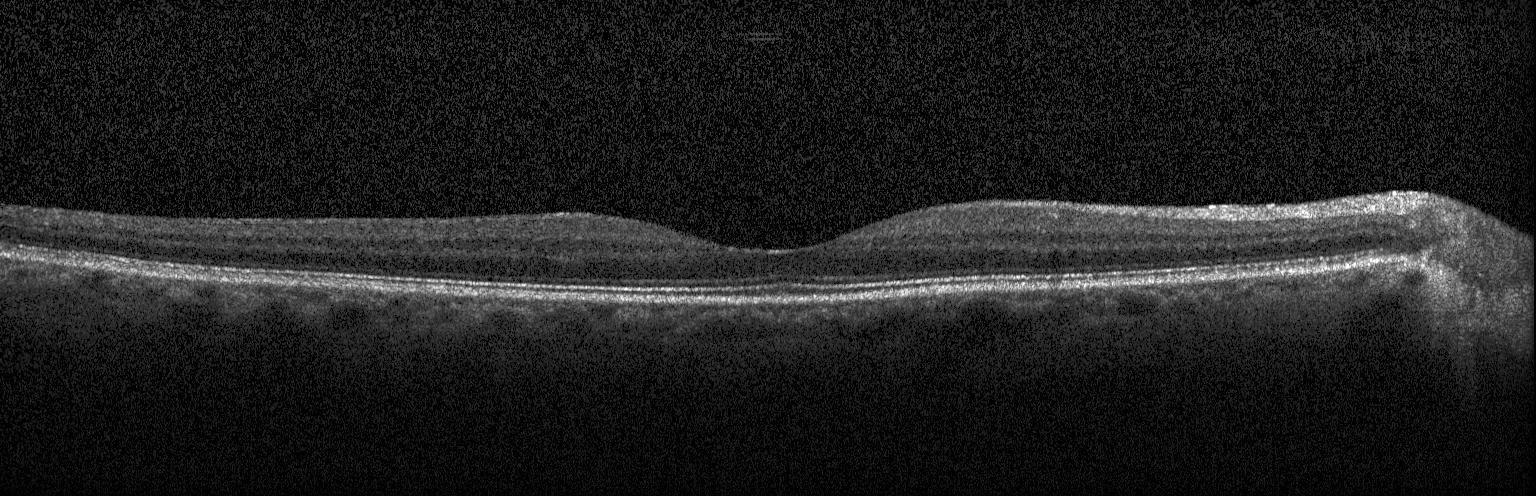
OCT B-scan
Assessment: no choroidal neovascularization, no diabetic macular edema, and no drusen.